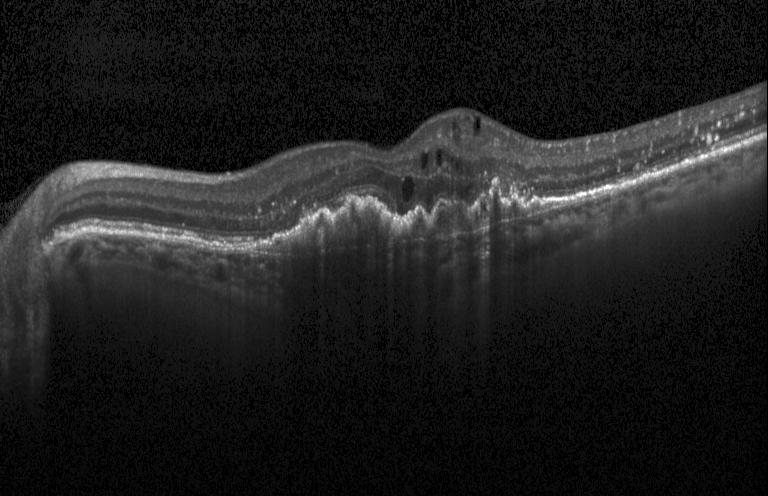
Spectral-domain OCT; retinal OCT cross-section; horizontal scan through the fovea.
Macular OCT: a choroidal neovascular membrane.